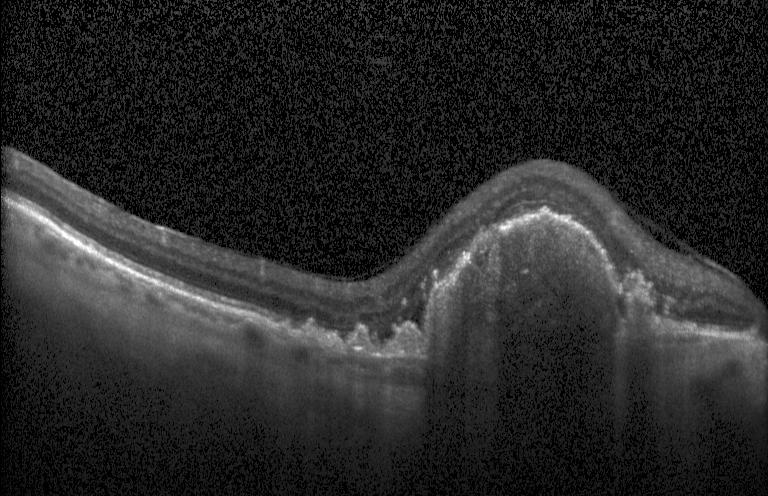 Finding: a choroidal neovascular membrane.